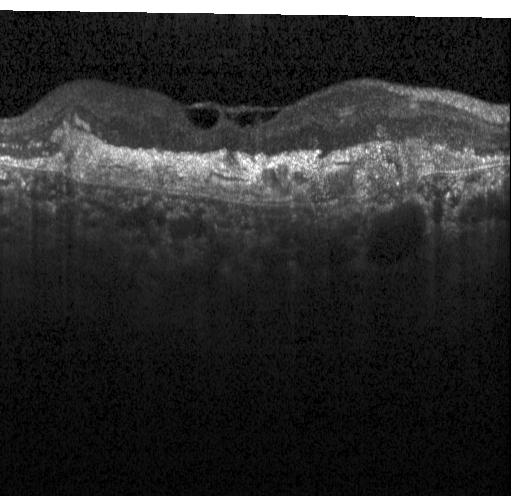 Retinal OCT B-scan — A choroidal neovascular membrane.